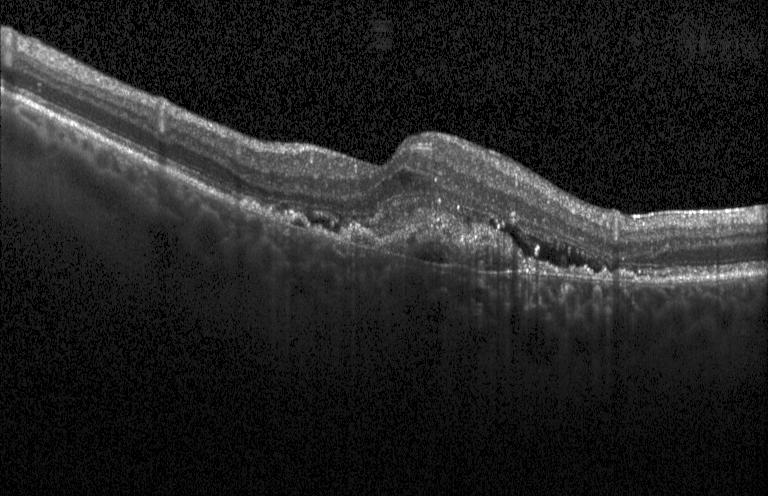
Retinal OCT cross-section
Diagnosis: a choroidal neovascular membrane.